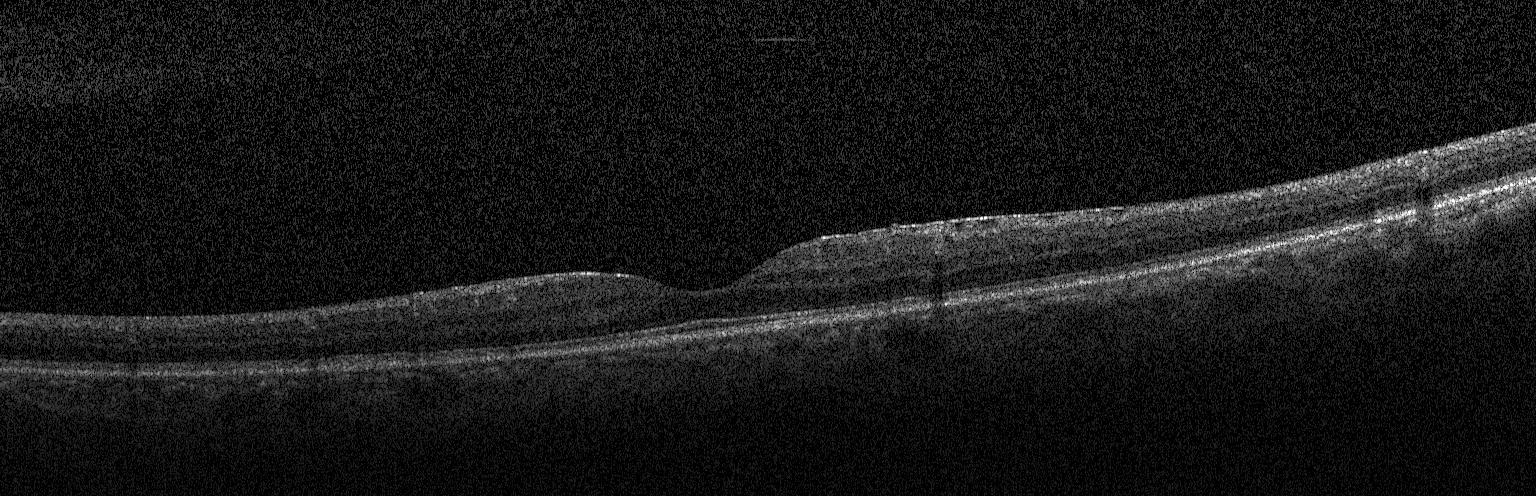 OCT line scan. Through the macula. Heidelberg Spectralis. SD-OCT — This B-scan demonstrates neither choroidal neovascularization, diabetic macular edema, nor drusen.